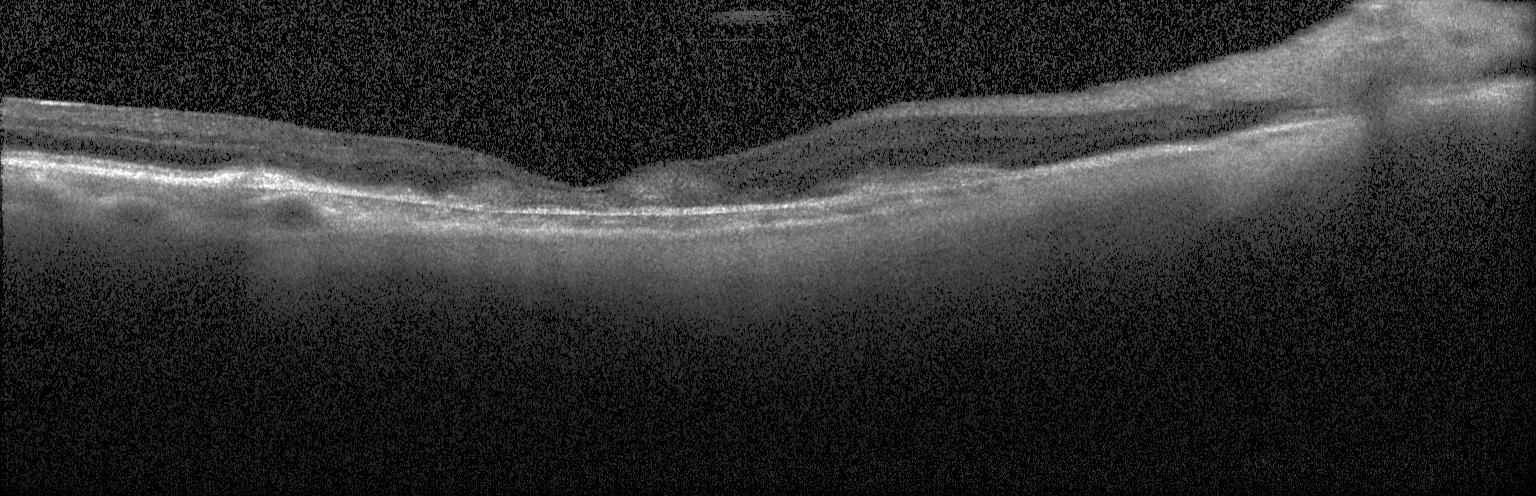

Macular OCT: a choroidal neovascular membrane.